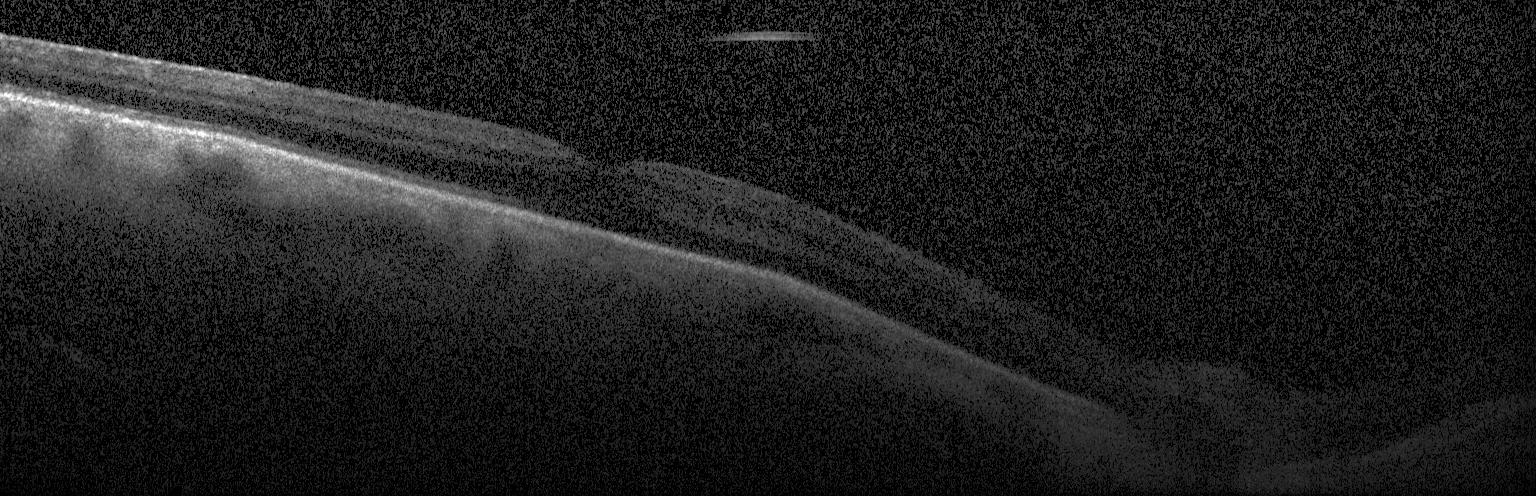

Neither choroidal neovascularization, diabetic macular edema, nor drusen.